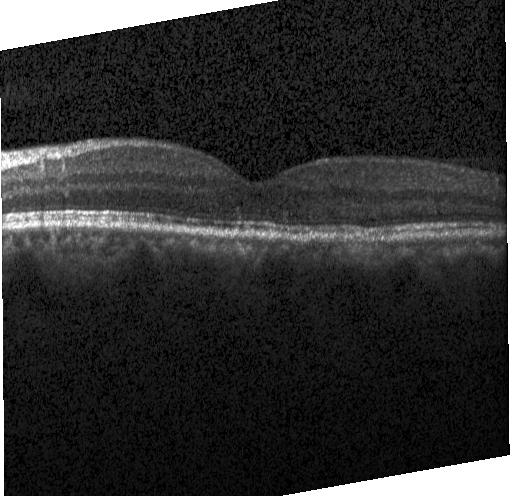

Retinal OCT B-scan — Assessment: no evidence of choroidal neovascularization, diabetic macular edema, or drusen.